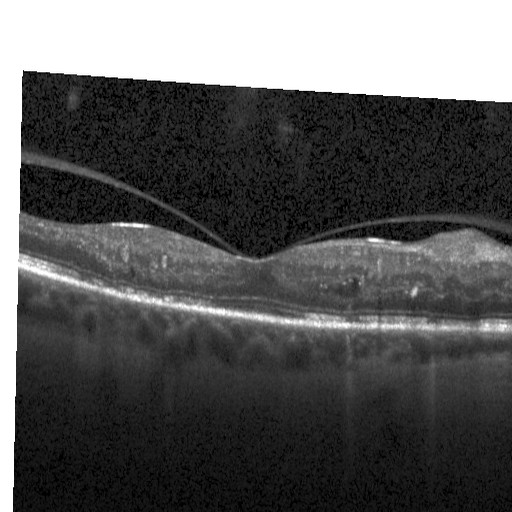
Instrument: Heidelberg Spectralis, optical coherence tomography B-scan, fovea-centered
Impression: diabetic macular edema.